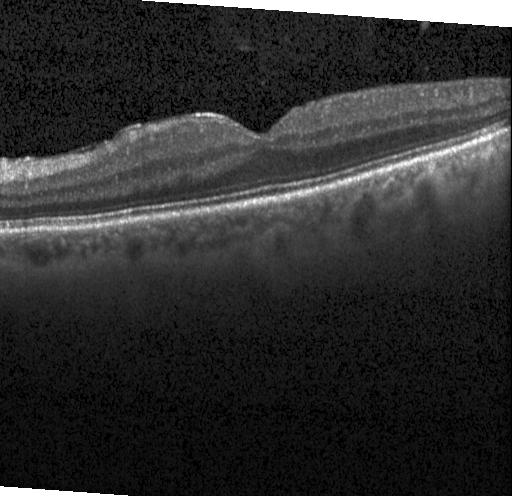

Optical coherence tomography B-scan; Heidelberg Spectralis; fovea-centered; spectral-domain optical coherence tomography. Impression: no evidence of choroidal neovascularization, diabetic macular edema, or drusen.